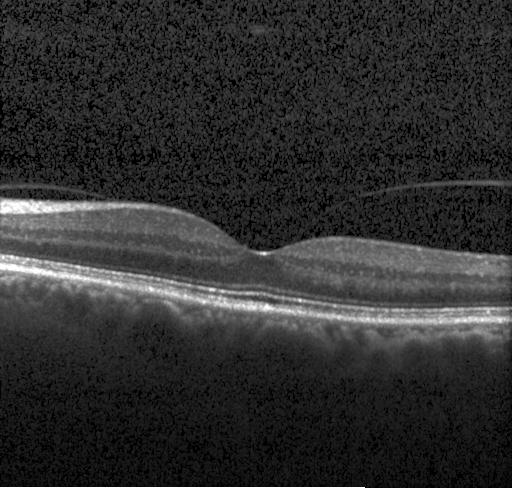 Instrument: Heidelberg Spectralis. Macular scan. SD-OCT. Retinal OCT B-scan — No evidence of CNV, DME, or drusen.